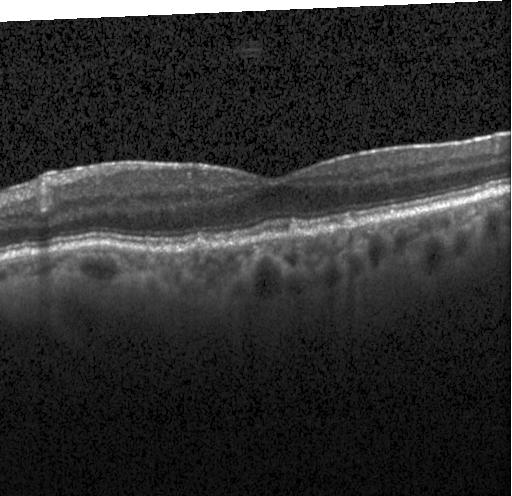 SD-OCT, OCT B-scan
Dx: multiple drusen.